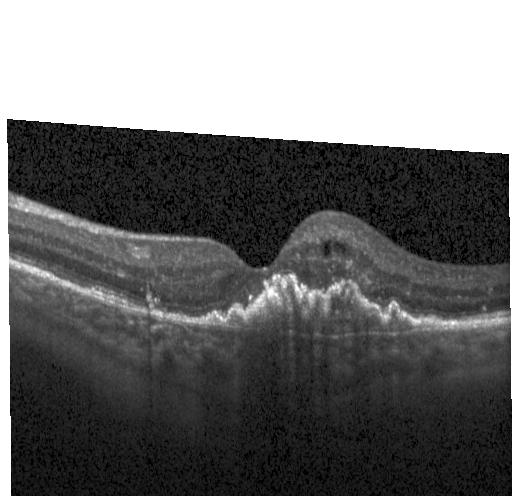

Fovea-centered; instrument: Heidelberg Spectralis; spectral-domain optical coherence tomography; optical coherence tomography scan.
Diagnosis: a choroidal neovascular membrane.